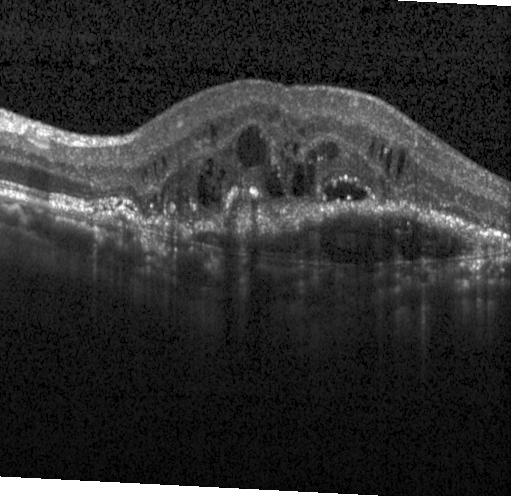

Macular OCT: CNV.